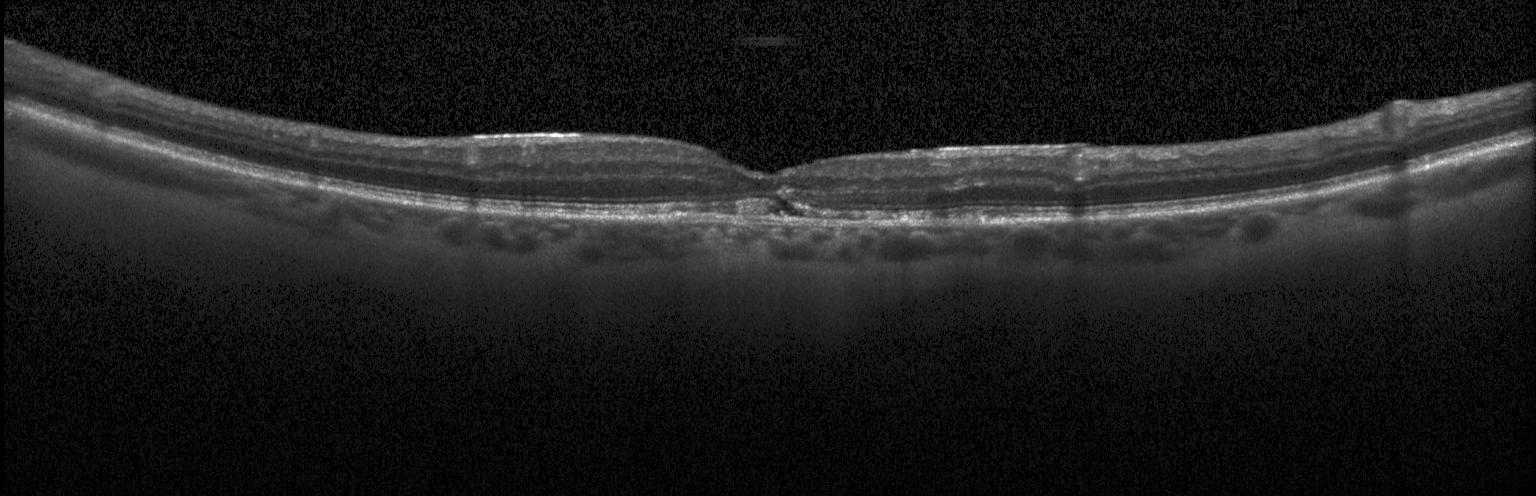

Spectral-domain optical coherence tomography, OCT B-scan. This B-scan demonstrates CNV.